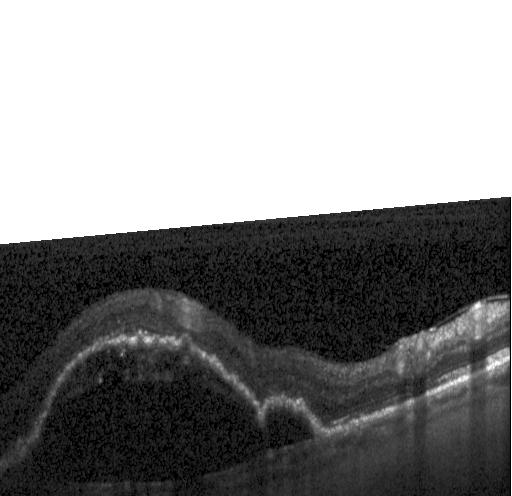 Optical coherence tomography B-scan; through the macula; instrument: Heidelberg Spectralis. Macular OCT: CNV.